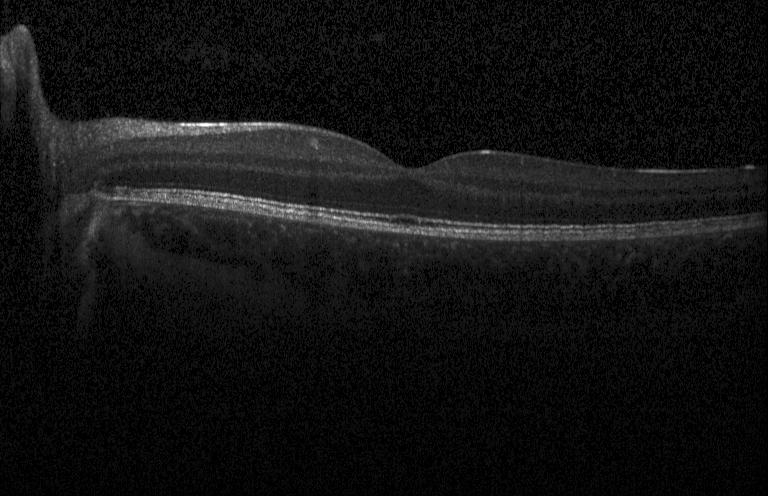 Horizontal scan through the fovea. Optical coherence tomography B-scan. Finding: no choroidal neovascularization, no diabetic macular edema, and no drusen.